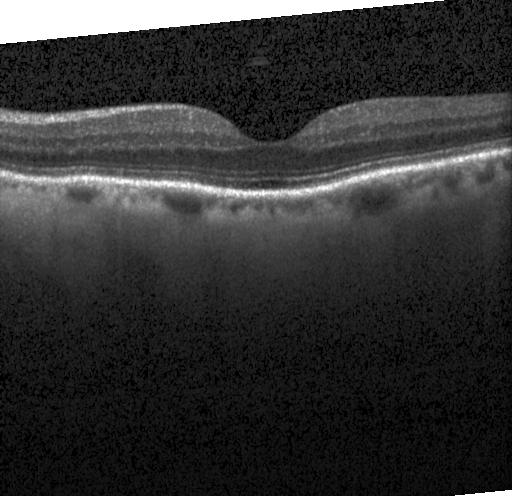
Finding: no evidence of choroidal neovascularization, diabetic macular edema, or drusen.